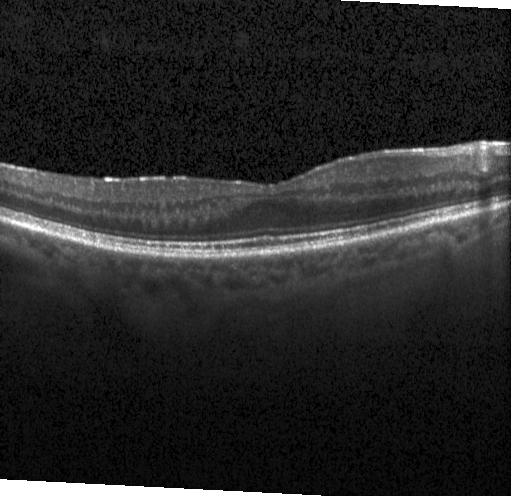
Finding: neither choroidal neovascularization, diabetic macular edema, nor drusen.